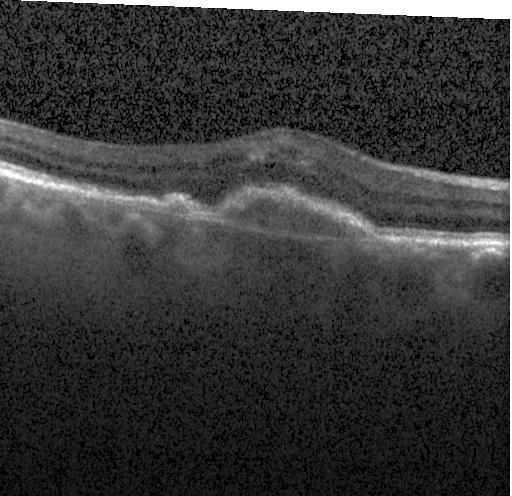
Heidelberg Spectralis OCT system, OCT line scan. Macular OCT: choroidal neovascularization (CNV).